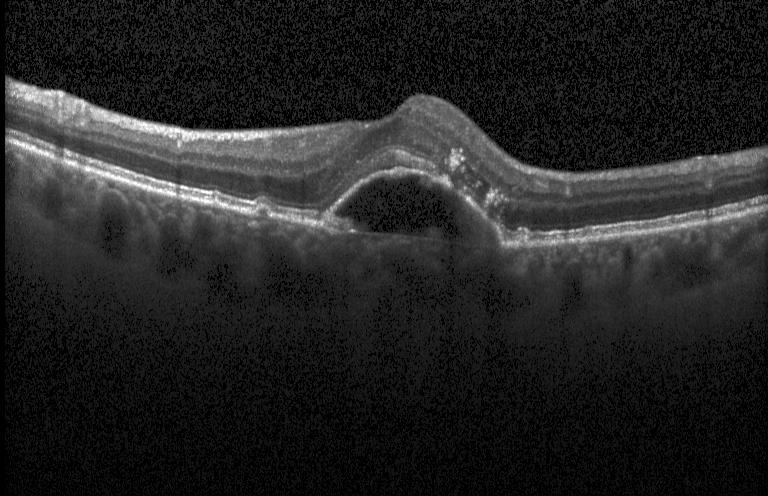
Optical coherence tomography B-scan, Heidelberg Spectralis OCT system
This B-scan demonstrates choroidal neovascularization.